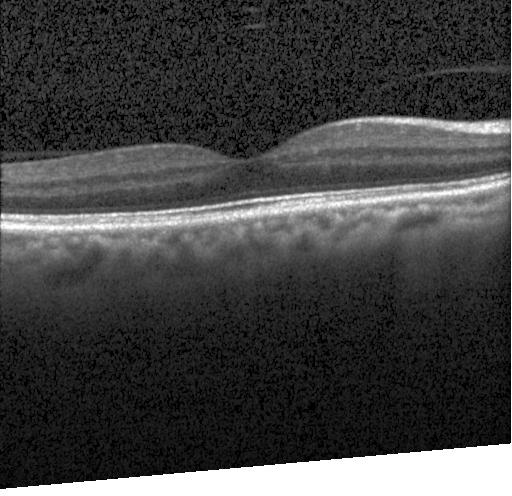
Assessment: no choroidal neovascularization, no diabetic macular edema, and no drusen.